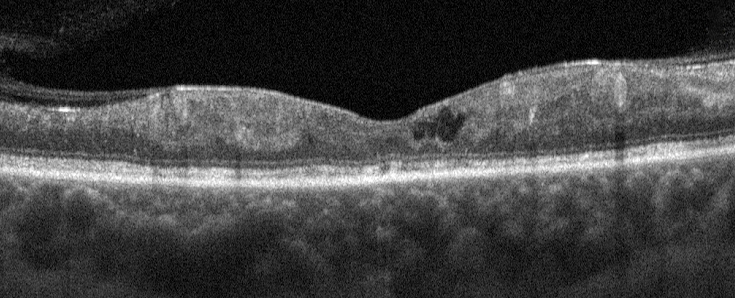 OCT line scan.
Assessment: diabetic macular edema (DME).